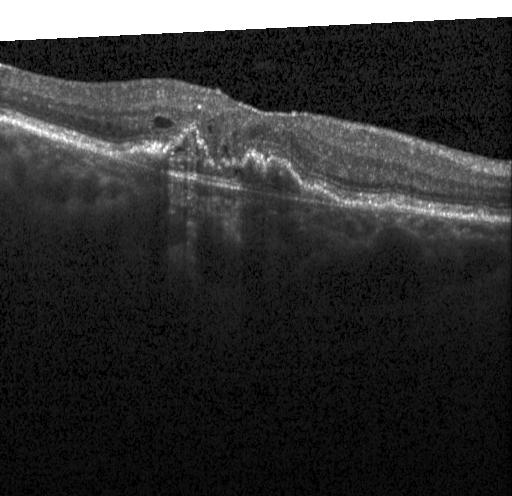 SD-OCT · retinal OCT cross-section. Choroidal neovascularization.